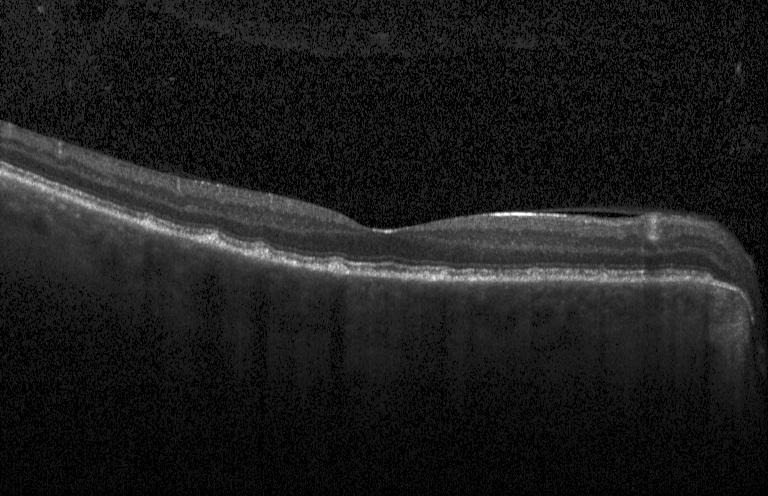

OCT finding: sub-RPE drusenoid deposits.